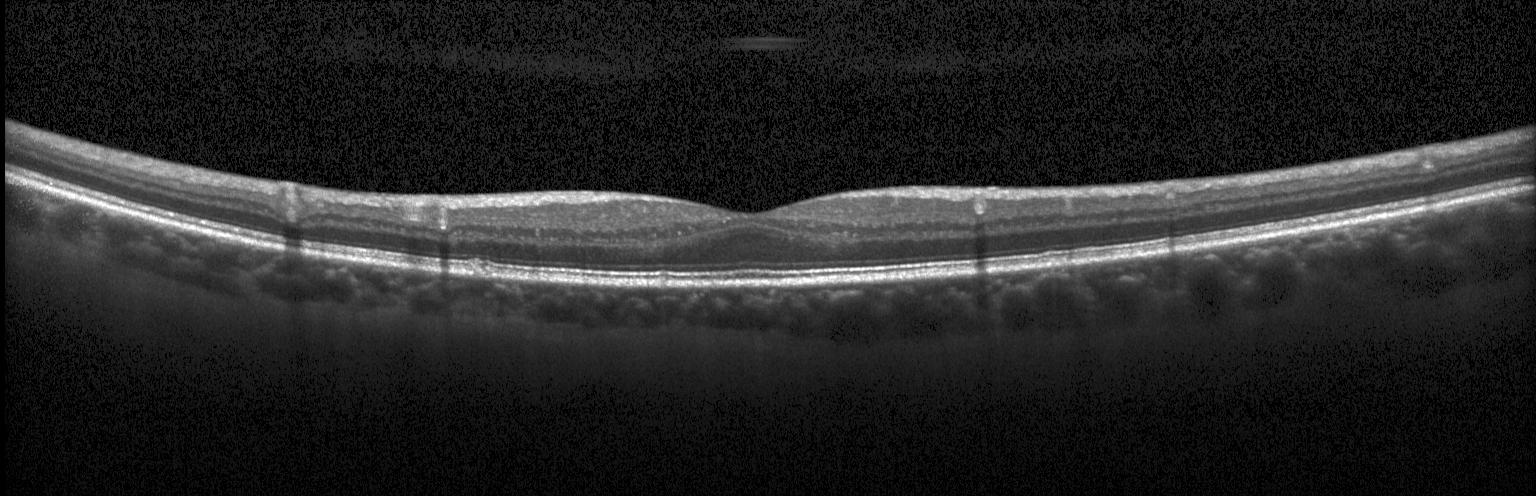
Optical coherence tomography scan; spectral-domain optical coherence tomography; through the macula; Heidelberg Spectralis.
Finding: no choroidal neovascularization, diabetic macular edema, or drusen.